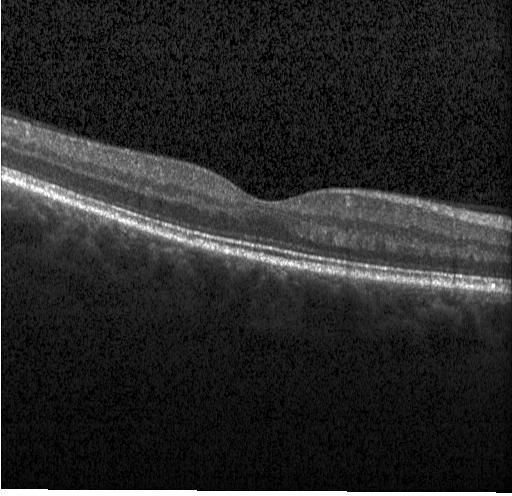

Spectral-domain optical coherence tomography · fovea-centered · retinal OCT cross-section.
Finding: neither choroidal neovascularization, diabetic macular edema, nor drusen.